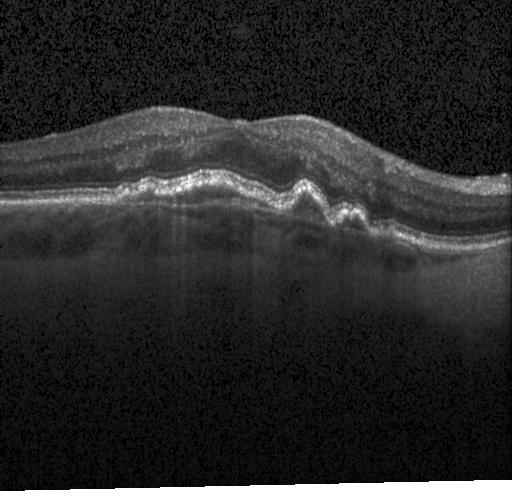 Diagnosis: choroidal neovascularization.